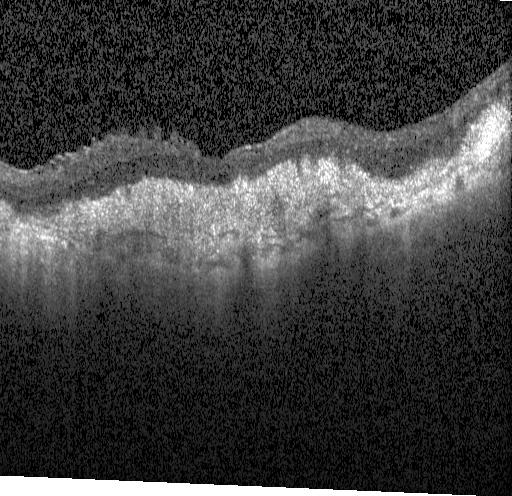

Centered on the fovea; retinal OCT cross-section — Diagnosis: choroidal neovascularization.